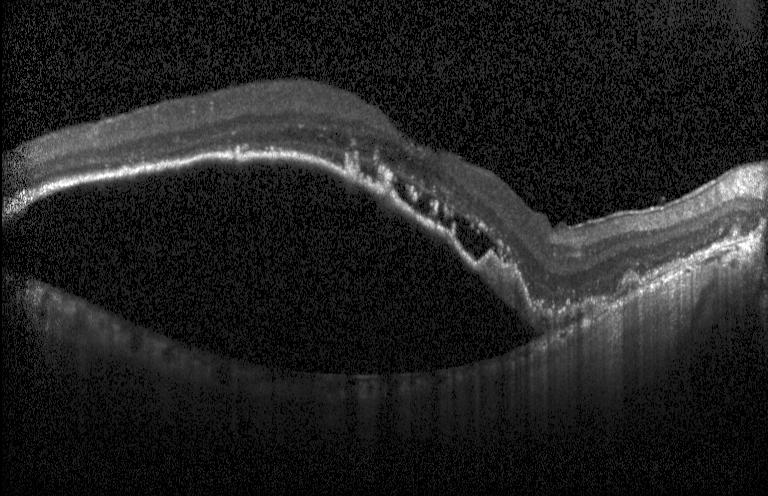

Heidelberg Spectralis OCT system, optical coherence tomography scan, horizontal scan through the fovea, spectral-domain OCT
Diagnosis: a choroidal neovascular membrane.